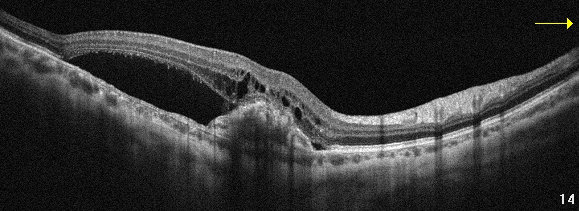

Retinal OCT cross-section, OD.
Impression: age-related macular degeneration (AMD).